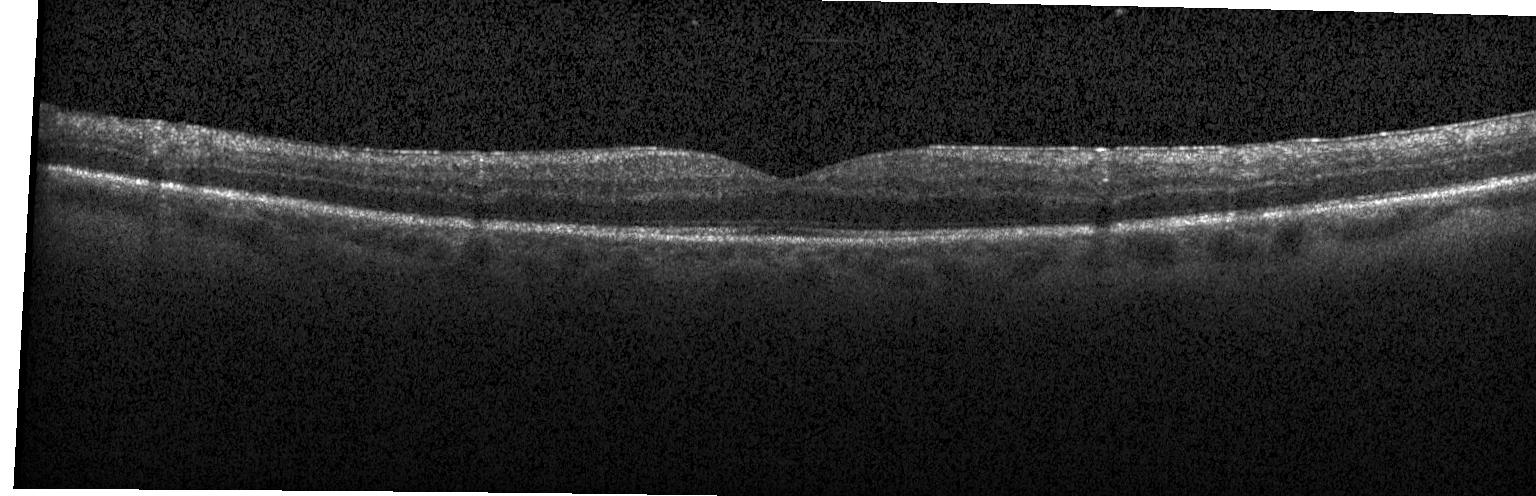 Retinal OCT B-scan.
Finding: no evidence of CNV, DME, or drusen.